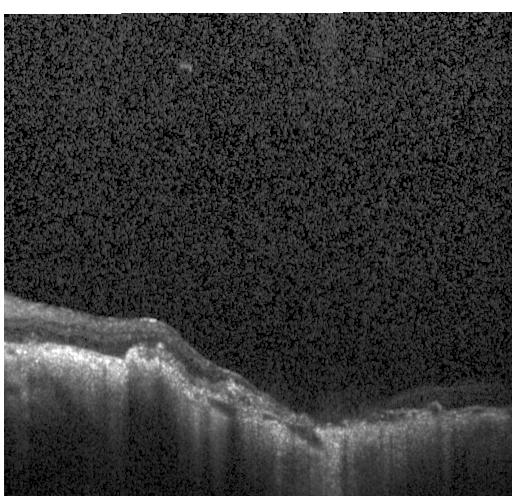
Finding: choroidal neovascularization (CNV).